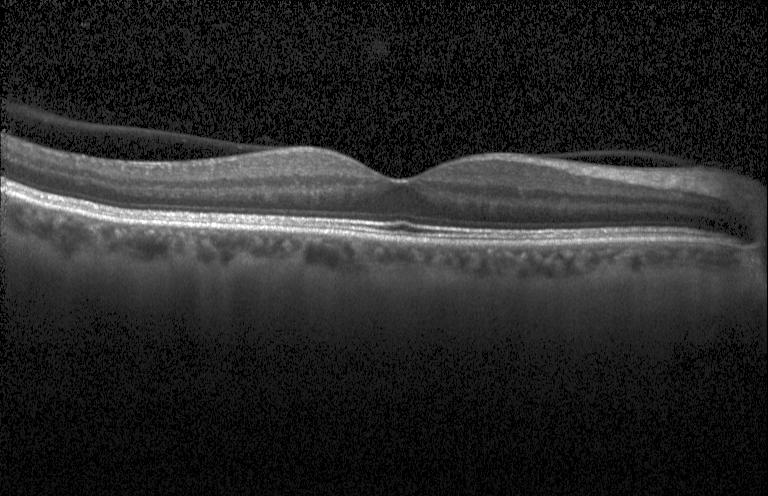
Optical coherence tomography scan. Impression: no CNV, DME, or drusen.